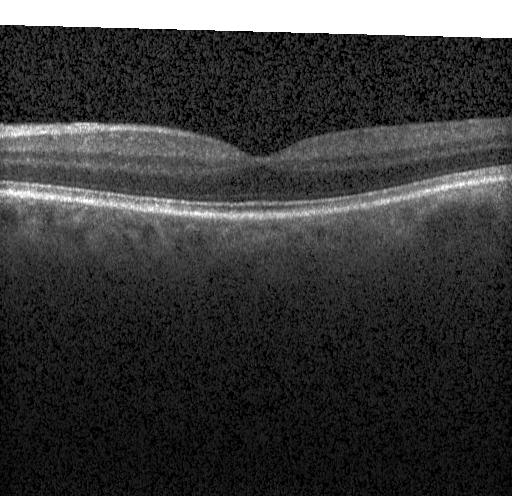
Optical coherence tomography scan.
Impression: no CNV, DME, or drusen.